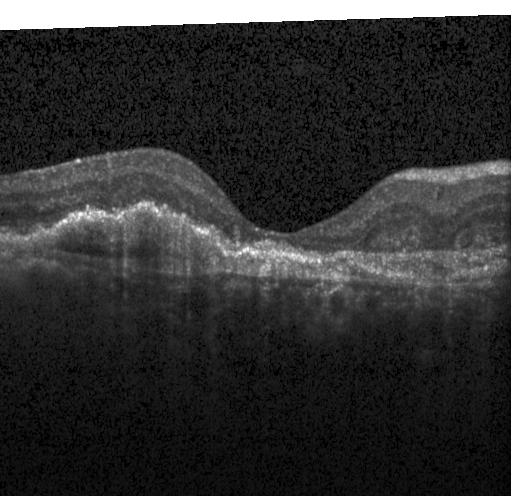 A choroidal neovascular membrane.